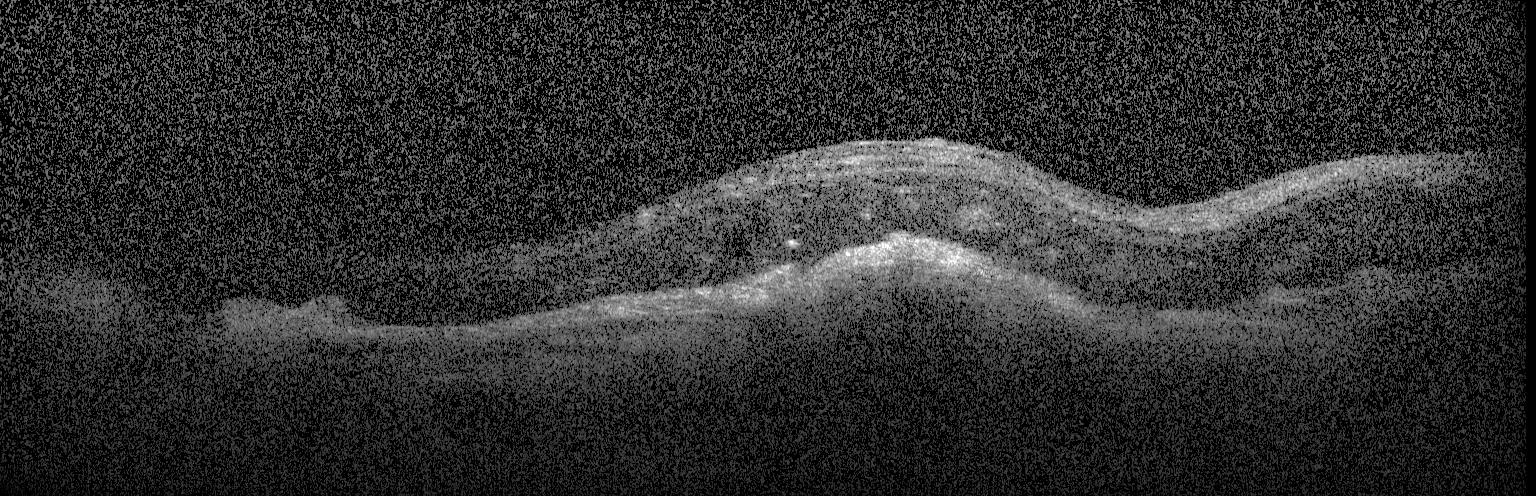 Heidelberg Spectralis, retinal OCT B-scan
Impression: a choroidal neovascular membrane.